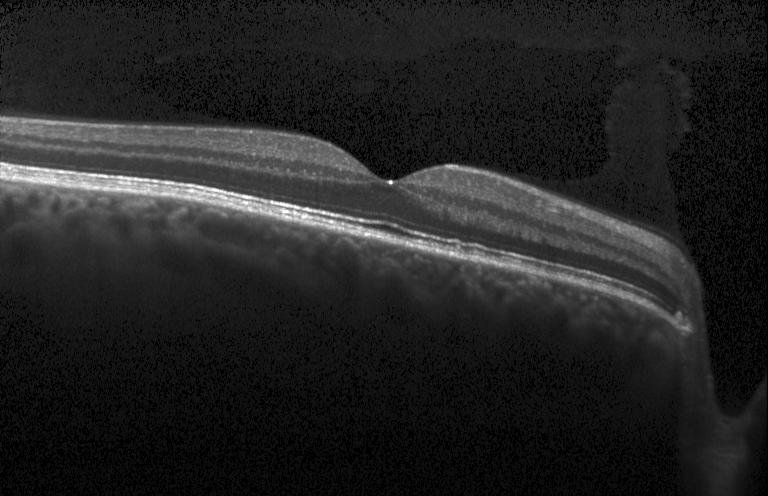 Diagnosis: no choroidal neovascularization, diabetic macular edema, or drusen.